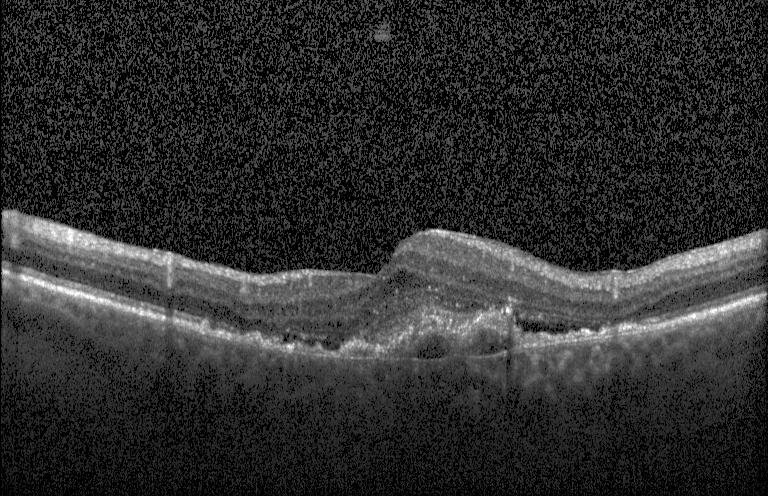 SD-OCT · optical coherence tomography B-scan
Impression: choroidal neovascularization.